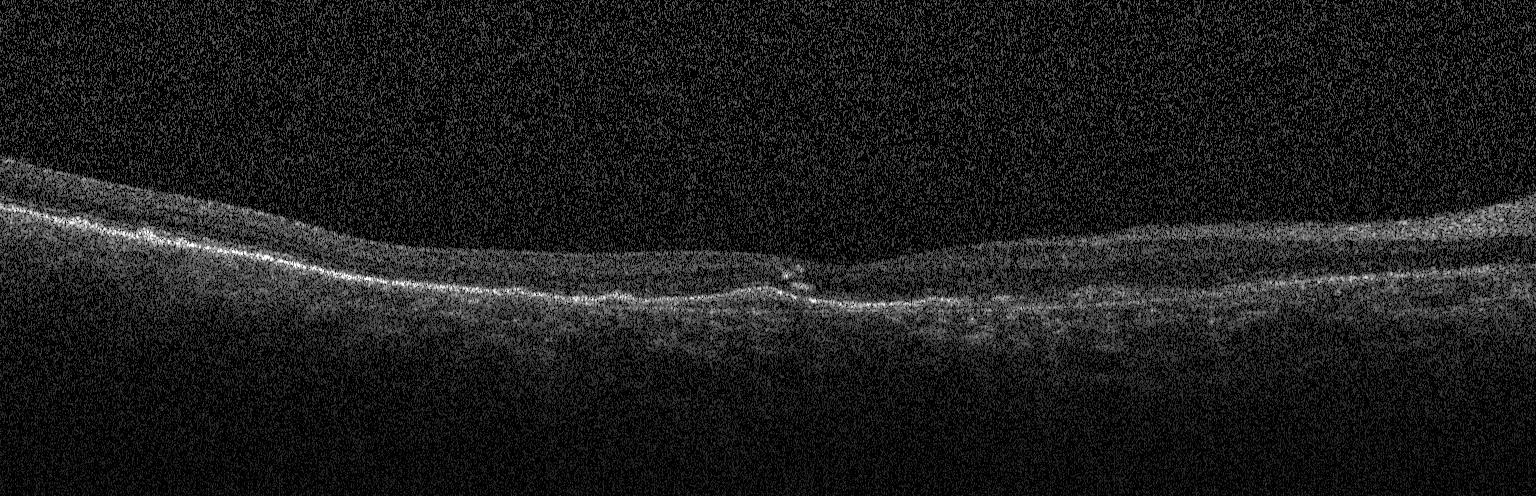

Spectral-domain optical coherence tomography, OCT B-scan, centered on the fovea.
Finding: a choroidal neovascular membrane.